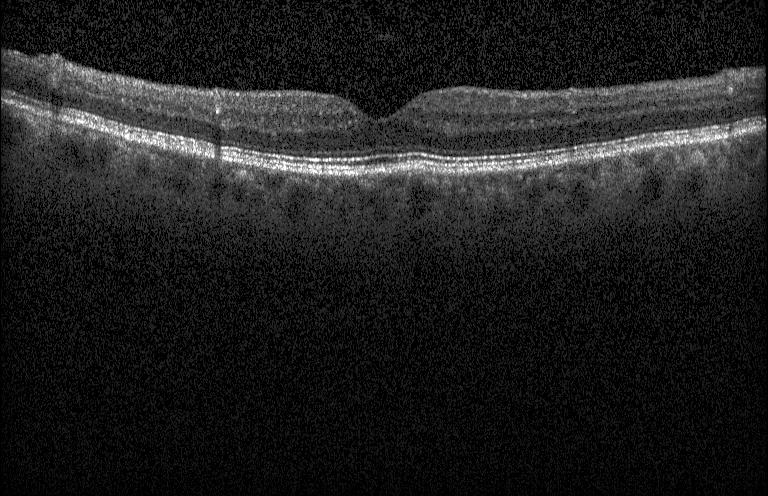 Through the macula · OCT B-scan
Diagnosis: neither choroidal neovascularization, diabetic macular edema, nor drusen.